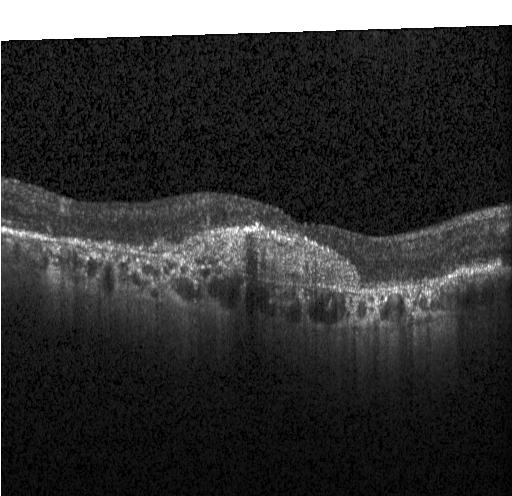

This B-scan demonstrates a choroidal neovascular membrane.